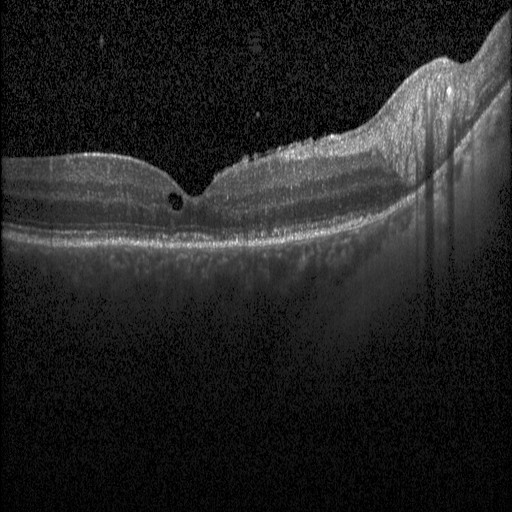 OCT B-scan; Heidelberg Spectralis OCT system. DME.